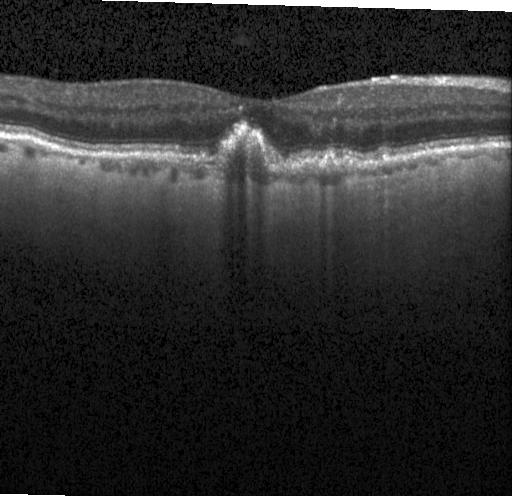

Diagnosis: multiple drusen.